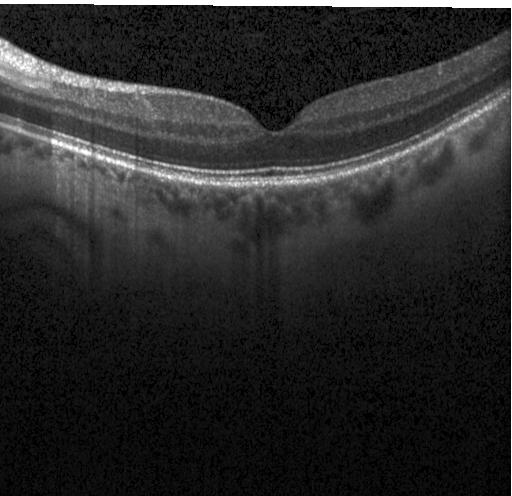 Assessment: no CNV, no DME, and no drusen.